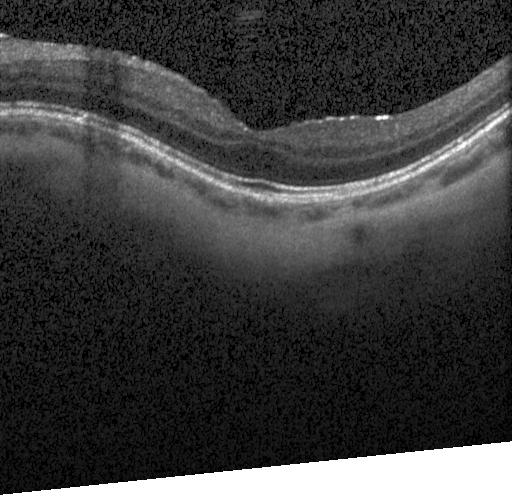

Retinal OCT cross-section showing neither choroidal neovascularization, diabetic macular edema, nor drusen.